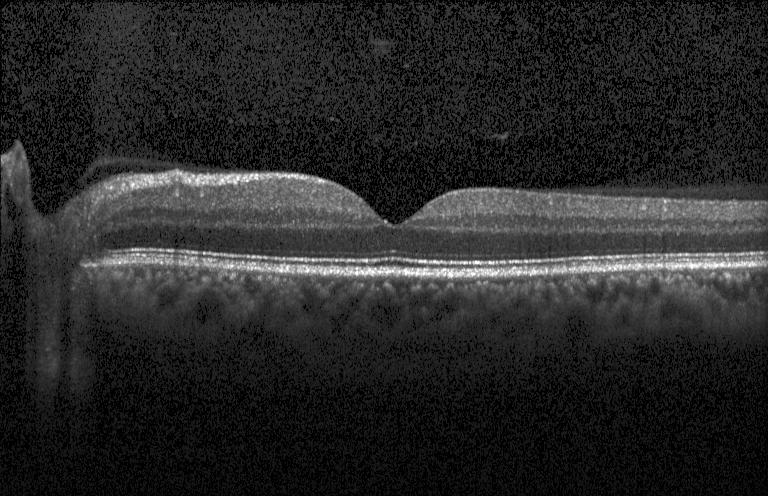
Macular scan. OCT B-scan. Acquired on a Heidelberg Spectralis — The scan shows no evidence of CNV, DME, or drusen.